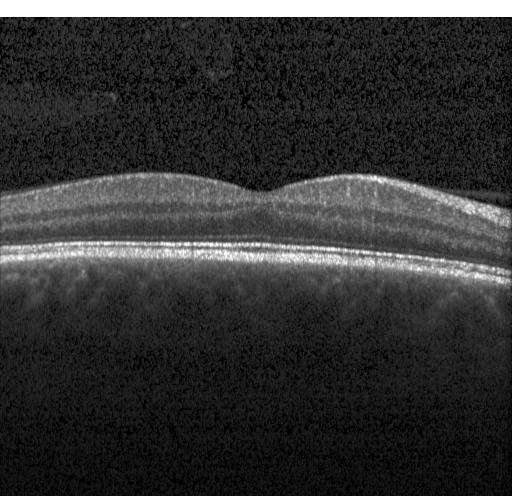 OCT line scan.
Assessment: no CNV, no DME, and no drusen.